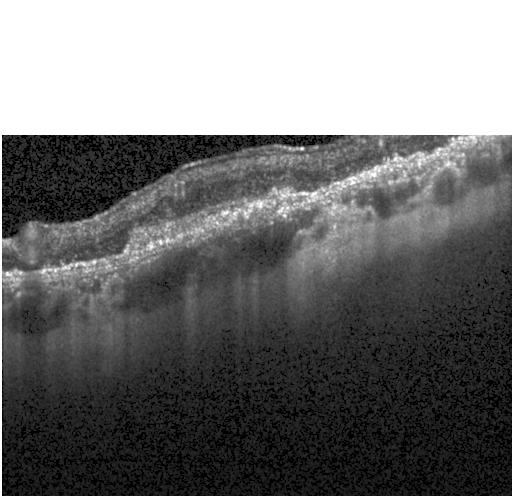
Retinal OCT cross-section. Acquired on a Heidelberg Spectralis. Diagnosis: CNV.